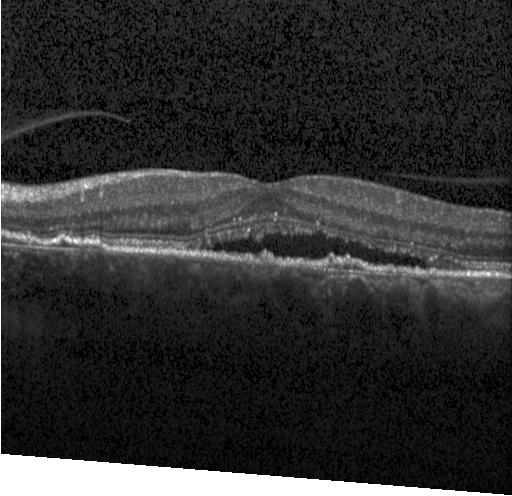 OCT finding: a choroidal neovascular membrane.